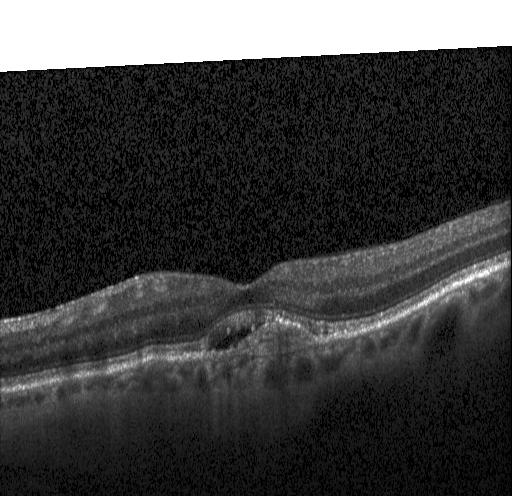

Impression: a choroidal neovascular membrane.